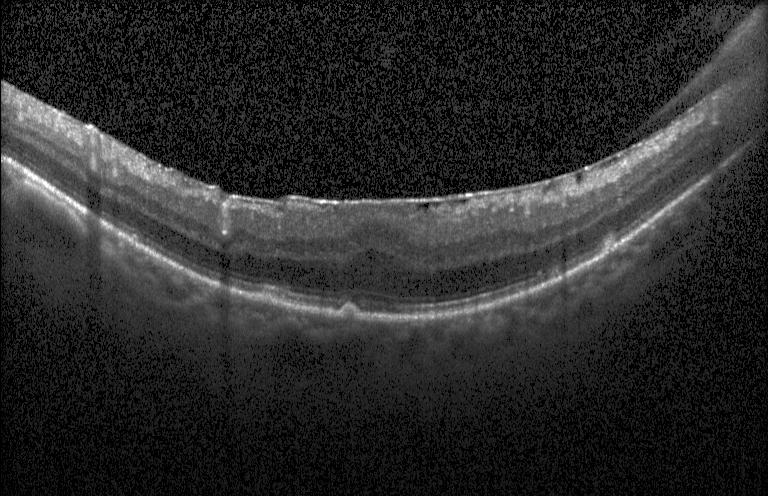
Retinal OCT cross-section — Assessment: sub-RPE drusenoid deposits.